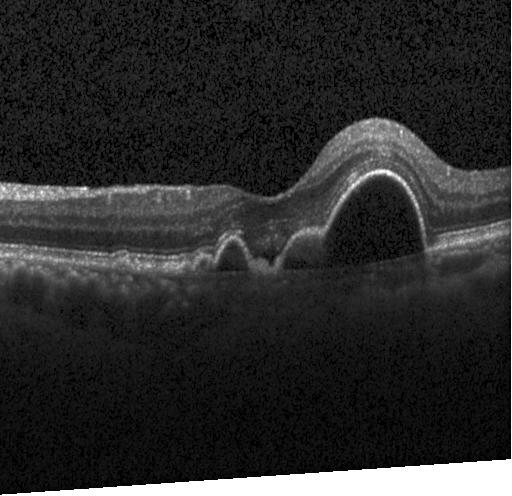
Spectral-domain OCT, retinal OCT cross-section, instrument: Heidelberg Spectralis. Finding: CNV.